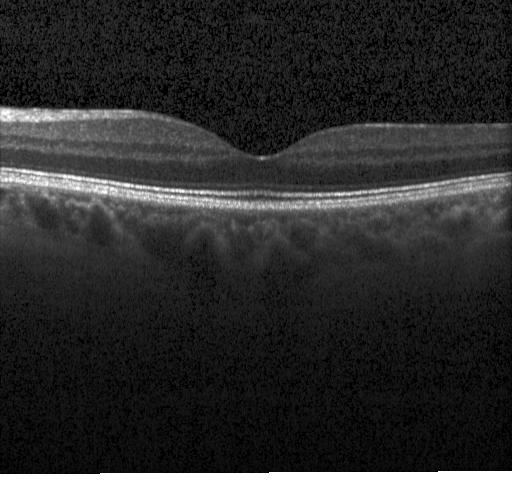 Spectral-domain OCT B-scan: neither choroidal neovascularization, diabetic macular edema, nor drusen.